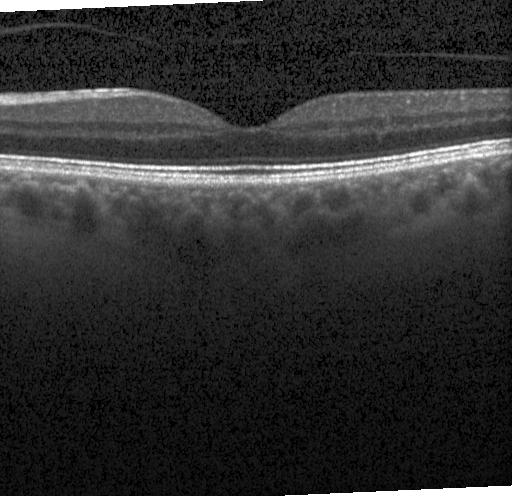

Dx: no evidence of choroidal neovascularization, diabetic macular edema, or drusen.